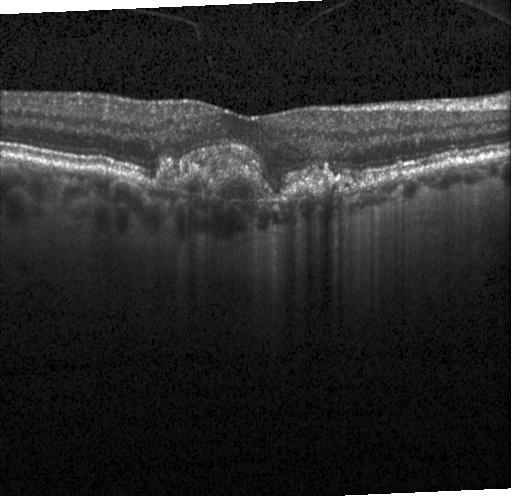
This B-scan demonstrates a choroidal neovascular membrane.